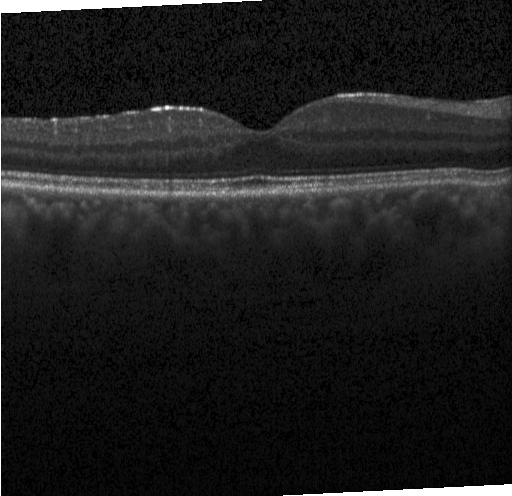

Diagnosis: no choroidal neovascularization, no diabetic macular edema, and no drusen.